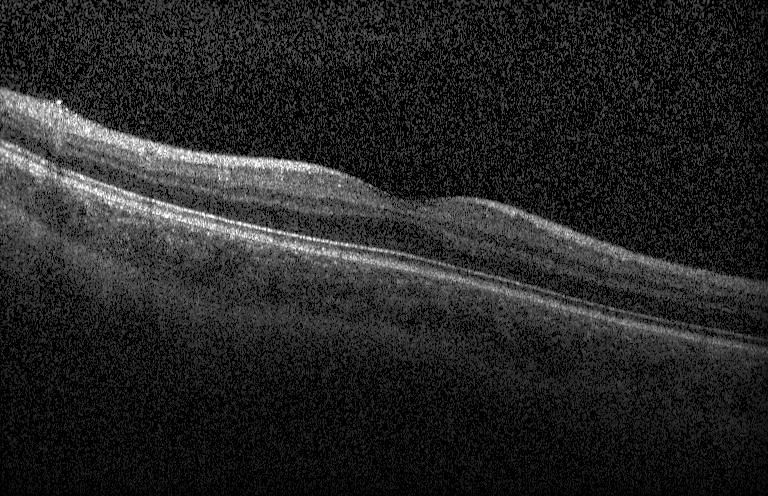

OCT scan showing no CNV, DME, or drusen.